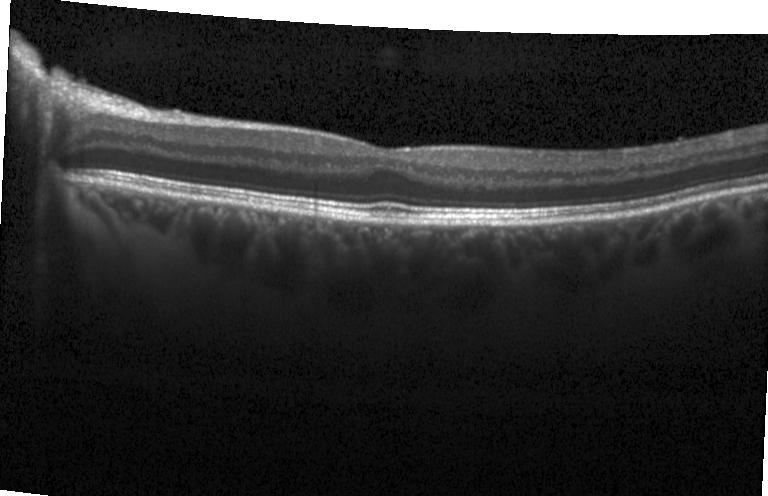
Impression: neither CNV, DME, nor drusen.